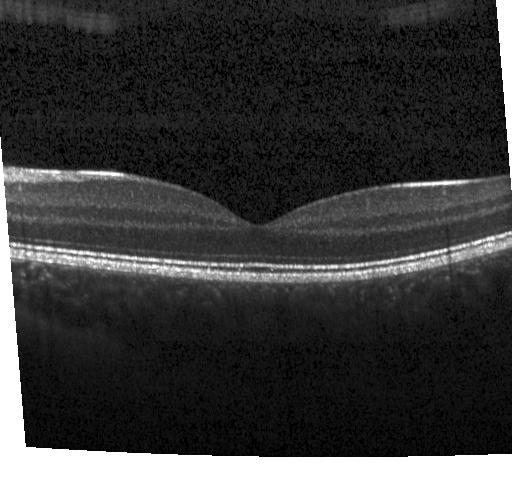

OCT line scan.
Dx: neither choroidal neovascularization, diabetic macular edema, nor drusen.